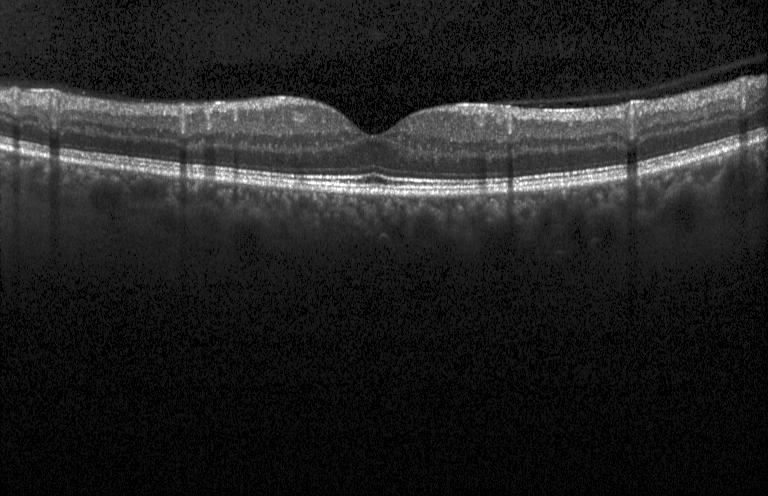

Macular scan. OCT B-scan. Spectral-domain OCT. The scan shows no choroidal neovascularization, diabetic macular edema, or drusen.